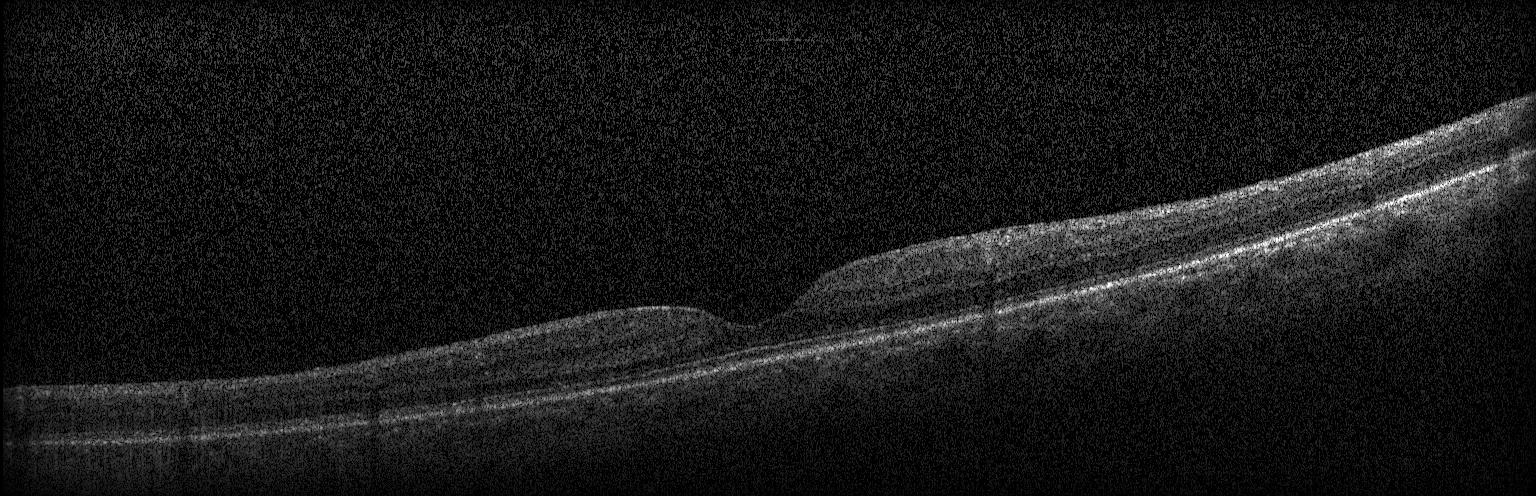
Spectral-domain OCT B-scan: no choroidal neovascularization, no diabetic macular edema, and no drusen.